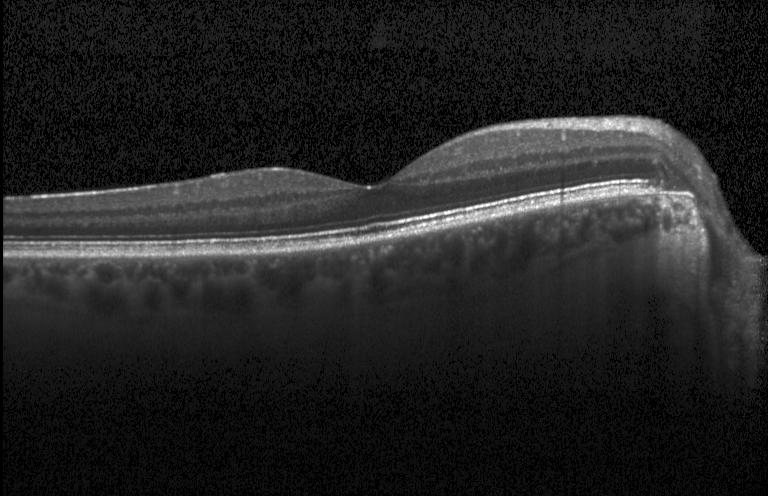
Neither CNV, DME, nor drusen.